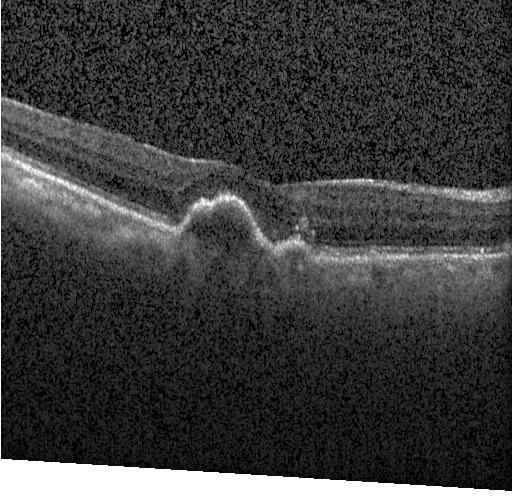

SD-OCT. Horizontal scan through the fovea. Optical coherence tomography B-scan
Impression: a choroidal neovascular membrane.